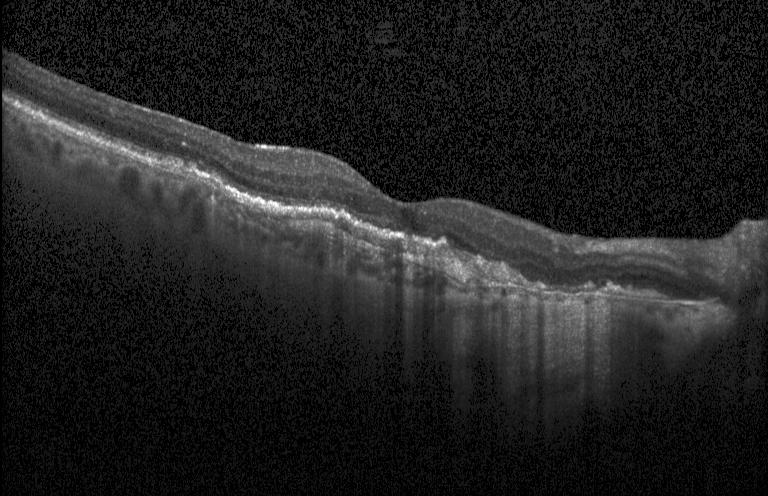

A choroidal neovascular membrane.